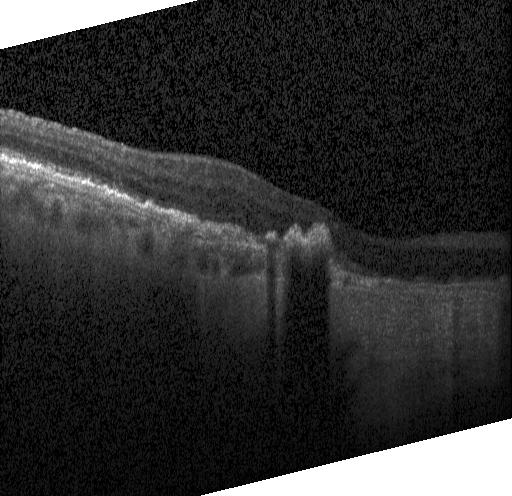

Centered on the fovea. Retinal OCT B-scan. Dx: a choroidal neovascular membrane.